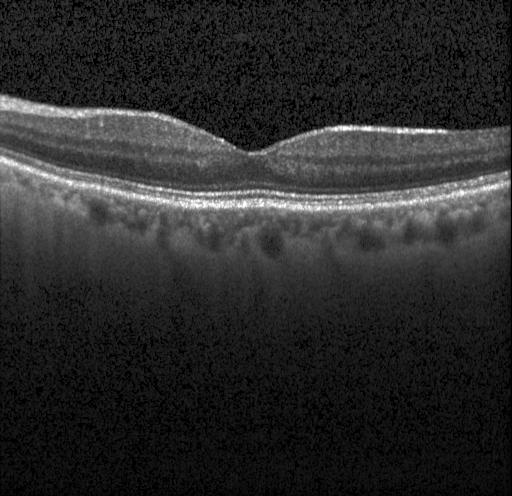 Heidelberg Spectralis, retinal OCT B-scan, horizontal scan through the fovea.
Impression: neither choroidal neovascularization, diabetic macular edema, nor drusen.